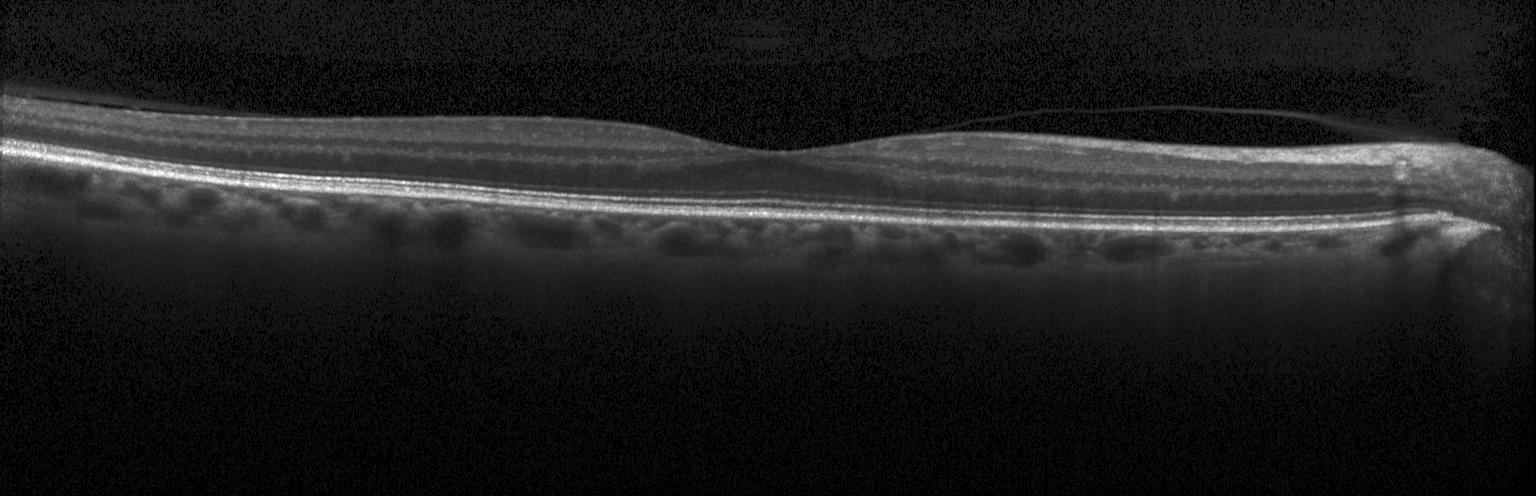

Finding: neither CNV, DME, nor drusen.